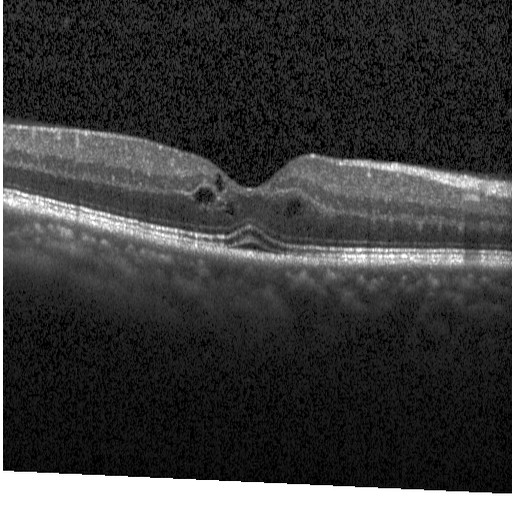
OCT line scan.
Finding: DME.